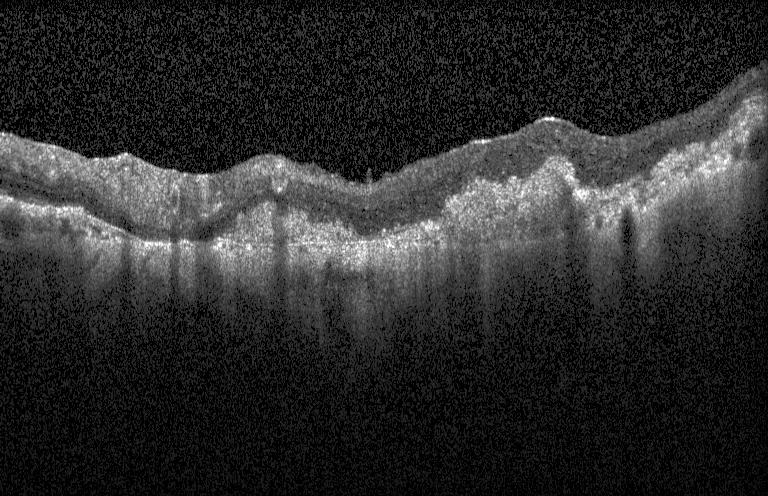

OCT finding: CNV.